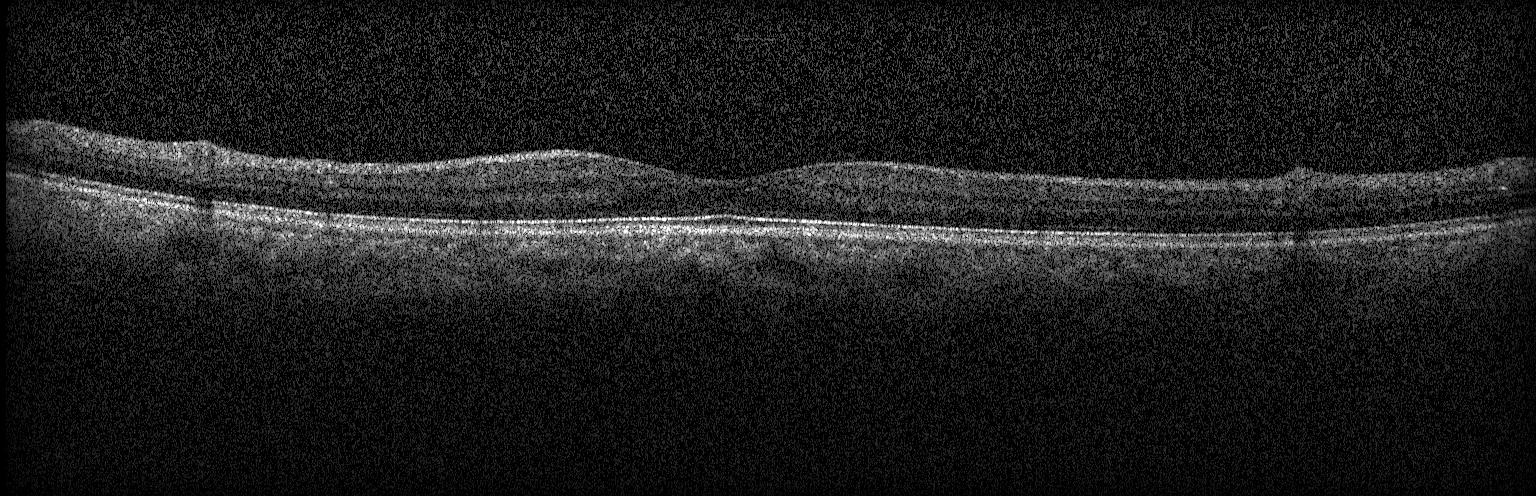
OCT B-scan. Impression: no choroidal neovascularization, diabetic macular edema, or drusen.